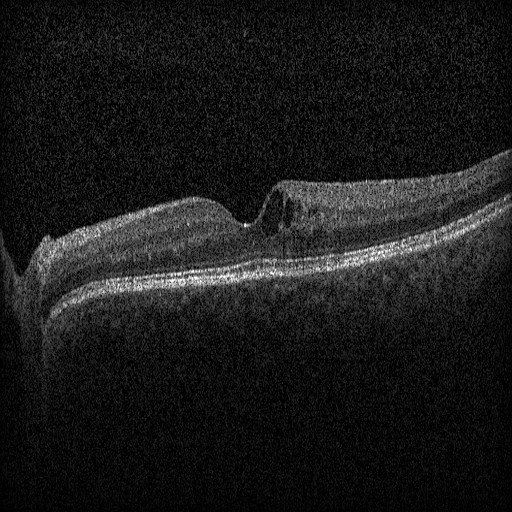 Macular scan; retinal OCT cross-section — OCT finding: diabetic macular edema (DME).